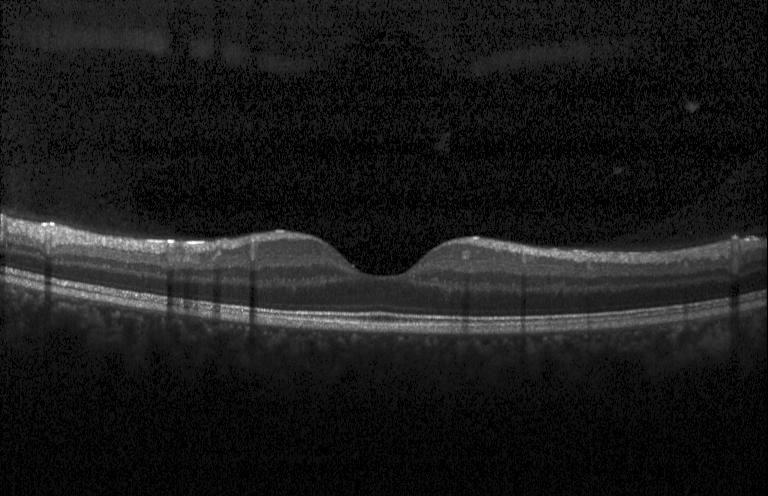

SD-OCT, OCT line scan, Heidelberg Spectralis OCT system
Diagnosis: no choroidal neovascularization, diabetic macular edema, or drusen.